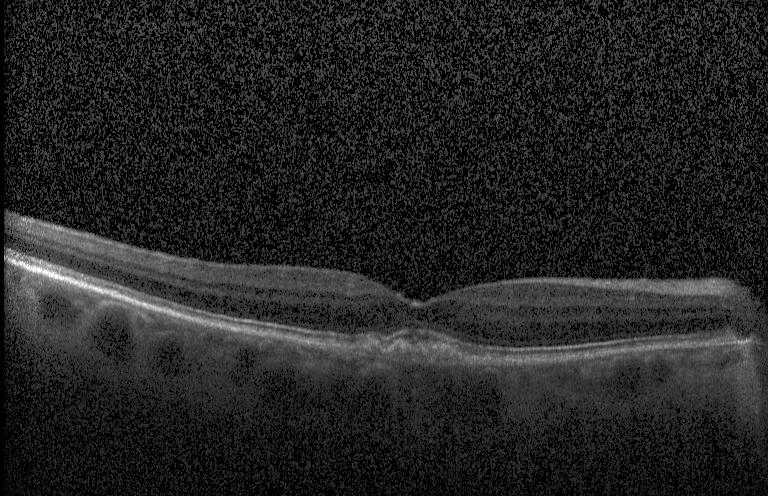

OCT line scan. Acquired on a Heidelberg Spectralis
The scan shows drusen.